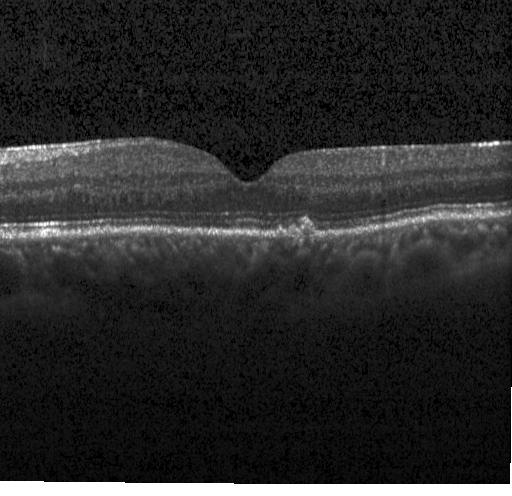 Fovea-centered. Instrument: Heidelberg Spectralis. OCT line scan. Finding: sub-RPE drusenoid deposits.